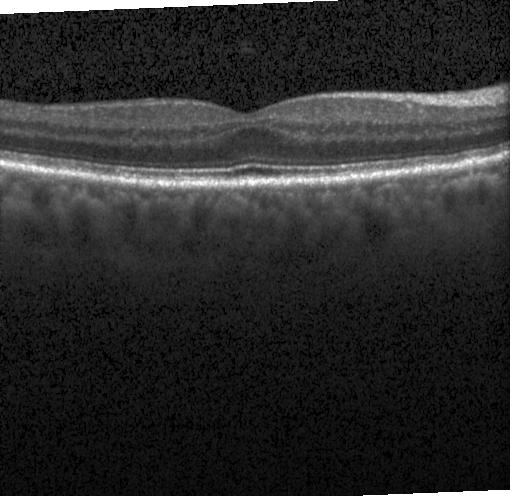
Optical coherence tomography scan. Heidelberg Spectralis OCT system.
This B-scan demonstrates no choroidal neovascularization, diabetic macular edema, or drusen.